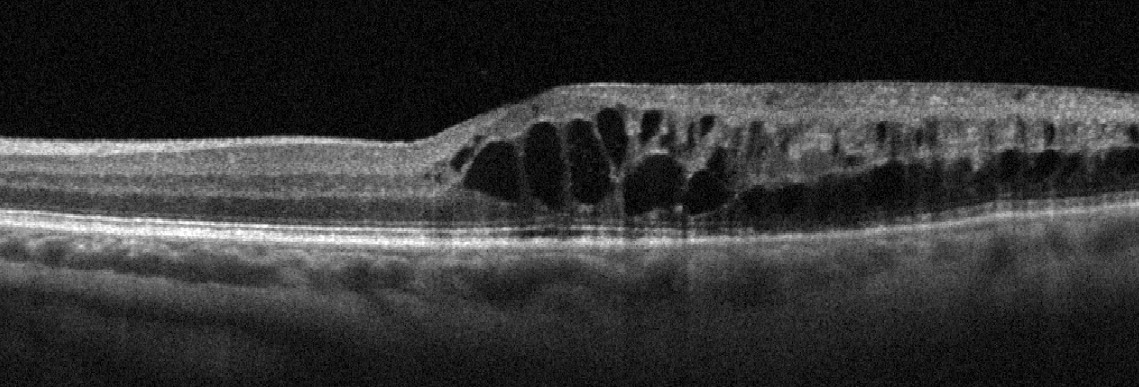 Diagnosis: retinal vein occlusion.